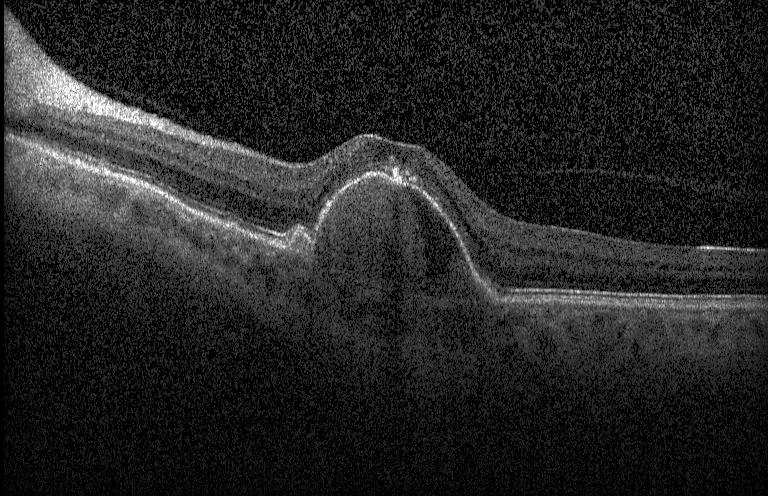
Heidelberg Spectralis. Spectral-domain OCT. Optical coherence tomography scan. A choroidal neovascular membrane.